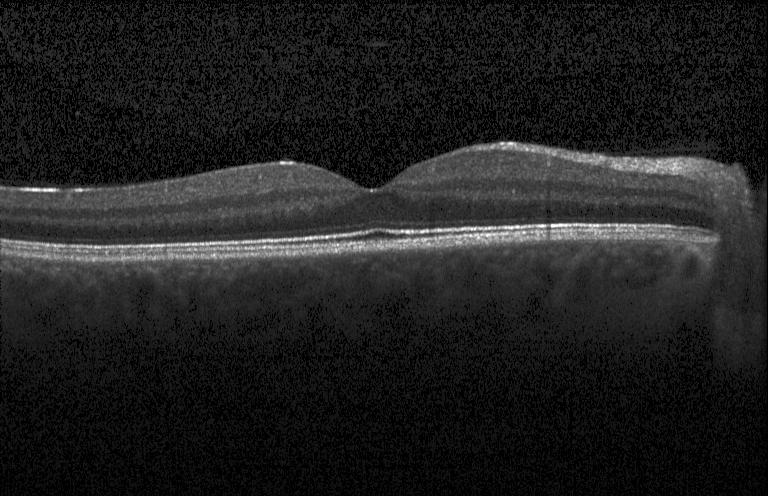
Retinal OCT cross-section; spectral-domain optical coherence tomography; Heidelberg Spectralis — No CNV, DME, or drusen.